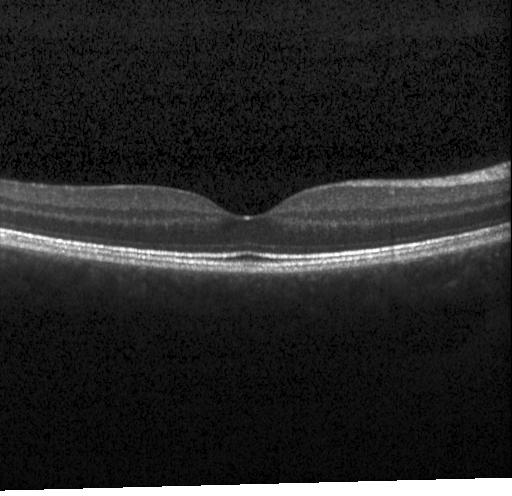
Horizontal scan through the fovea; optical coherence tomography B-scan; Heidelberg Spectralis; SD-OCT — Finding: no evidence of choroidal neovascularization, diabetic macular edema, or drusen.